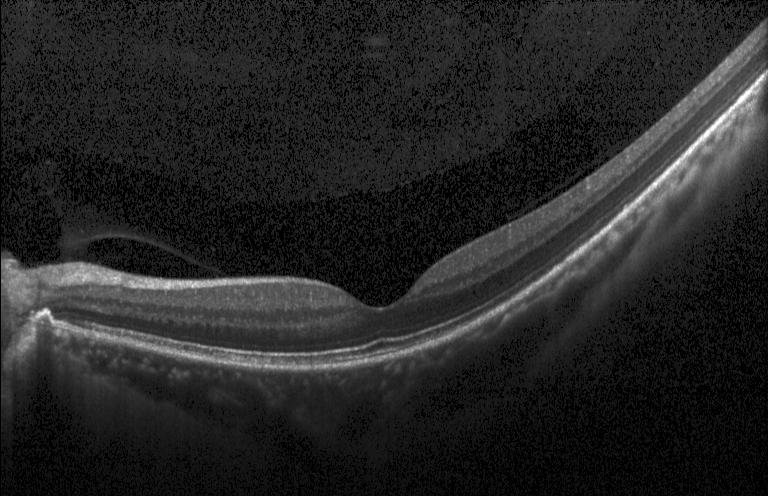 SD-OCT, instrument: Heidelberg Spectralis, optical coherence tomography scan
Impression: no evidence of choroidal neovascularization, diabetic macular edema, or drusen.